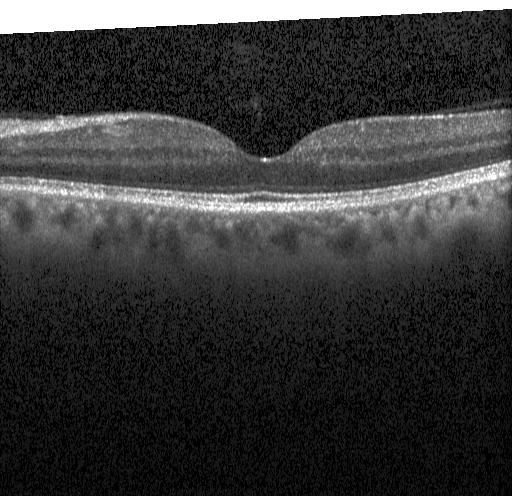

Retinal OCT cross-section showing no evidence of choroidal neovascularization, diabetic macular edema, or drusen.